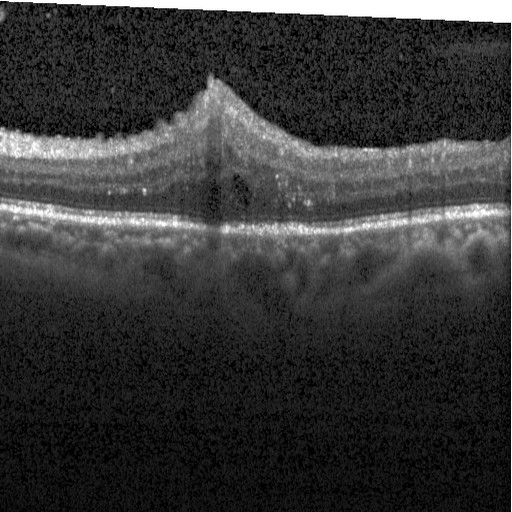

Assessment: diabetic macular edema.